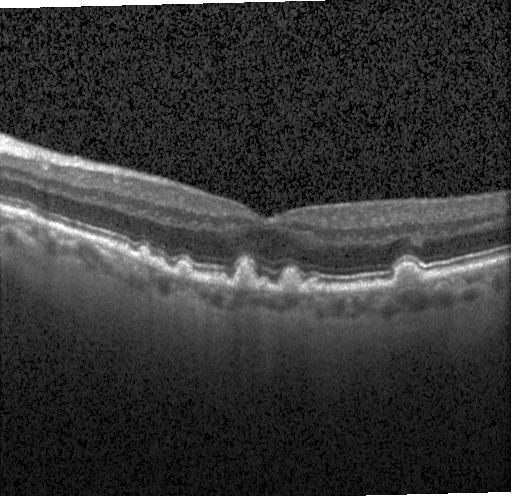 Instrument: Heidelberg Spectralis, spectral-domain optical coherence tomography, retinal OCT B-scan — This B-scan demonstrates sub-RPE drusenoid deposits.